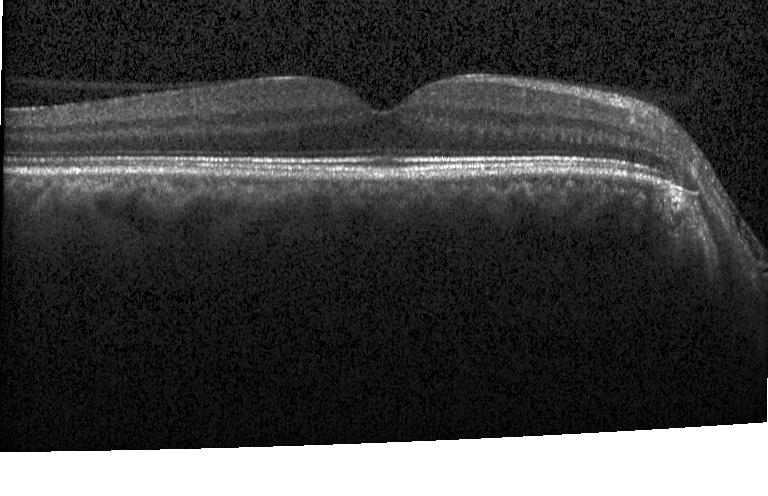
Heidelberg Spectralis. Spectral-domain optical coherence tomography. OCT line scan. Centered on the fovea.
Diagnosis: no choroidal neovascularization, no diabetic macular edema, and no drusen.